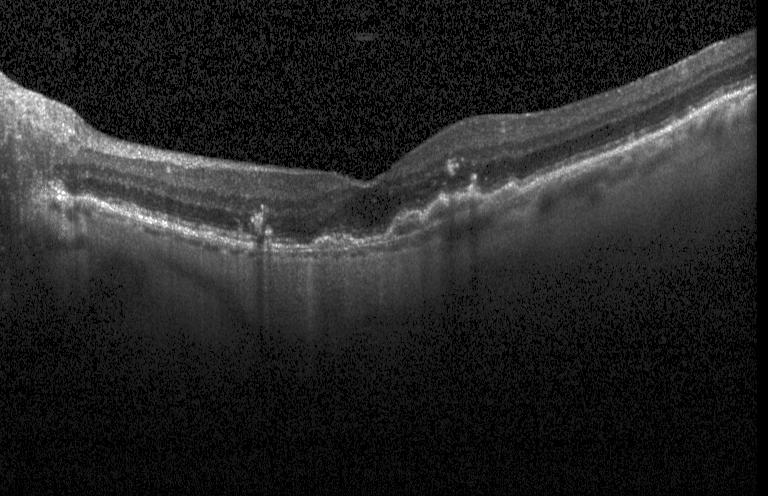
Spectral-domain OCT. Optical coherence tomography scan
CNV.